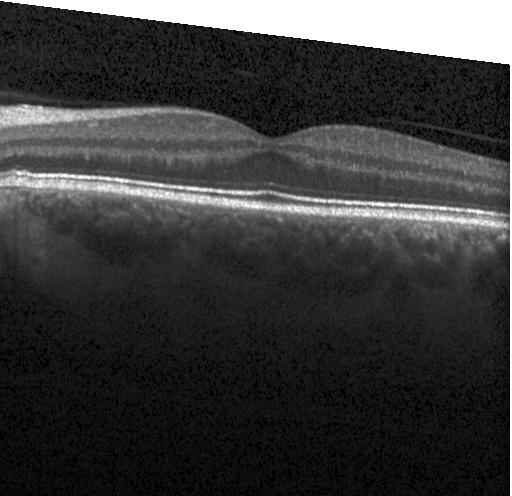
Impression: no choroidal neovascularization, diabetic macular edema, or drusen.